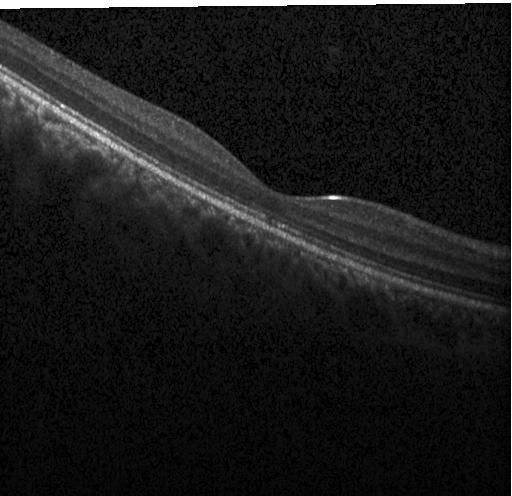 OCT finding: no choroidal neovascularization, no diabetic macular edema, and no drusen.